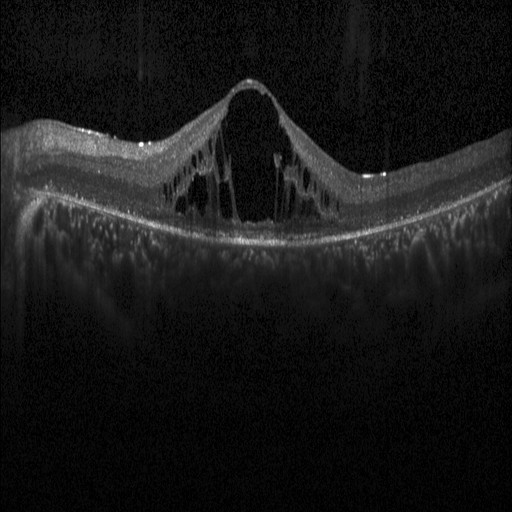

OCT line scan. Diagnosis: diabetic macular edema.